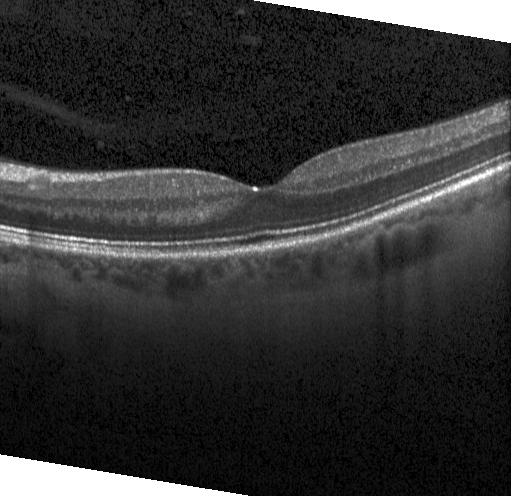

Acquired on a Heidelberg Spectralis, retinal OCT cross-section, horizontal scan through the fovea, spectral-domain OCT. Dx: no CNV, DME, or drusen.